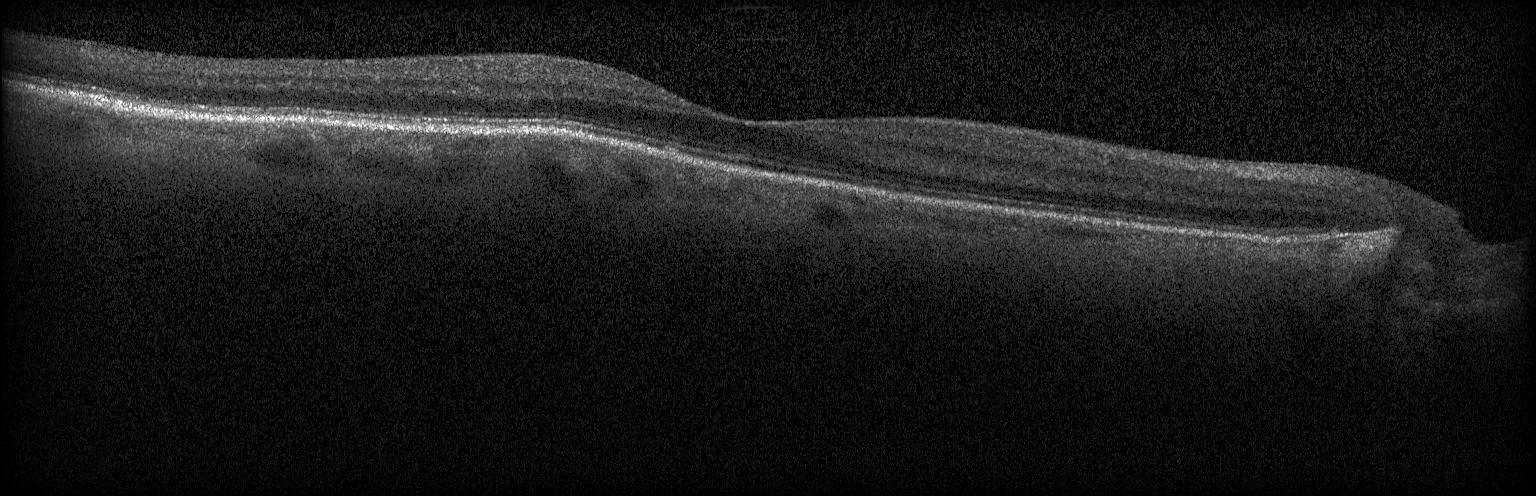

No choroidal neovascularization, diabetic macular edema, or drusen.